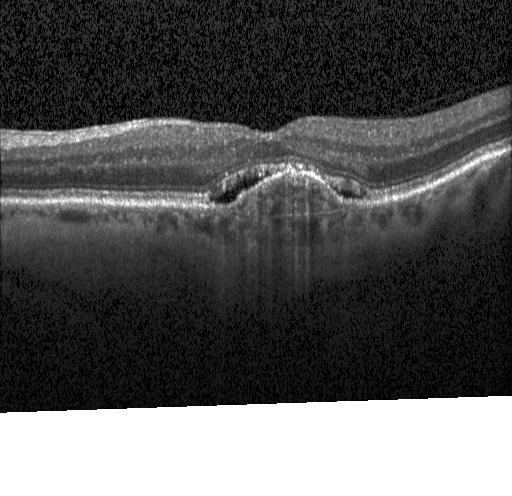
Optical coherence tomography B-scan; Heidelberg Spectralis OCT system; macular scan — Impression: choroidal neovascularization (CNV).